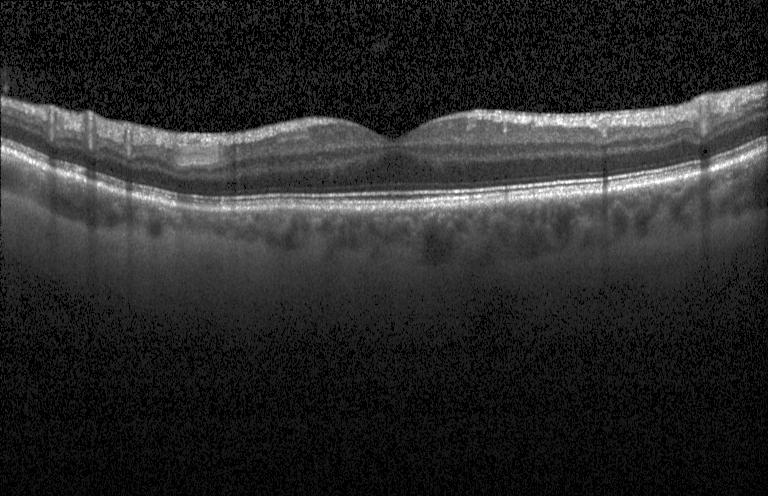

Through the macula · OCT line scan · Heidelberg Spectralis
Impression: no evidence of choroidal neovascularization, diabetic macular edema, or drusen.